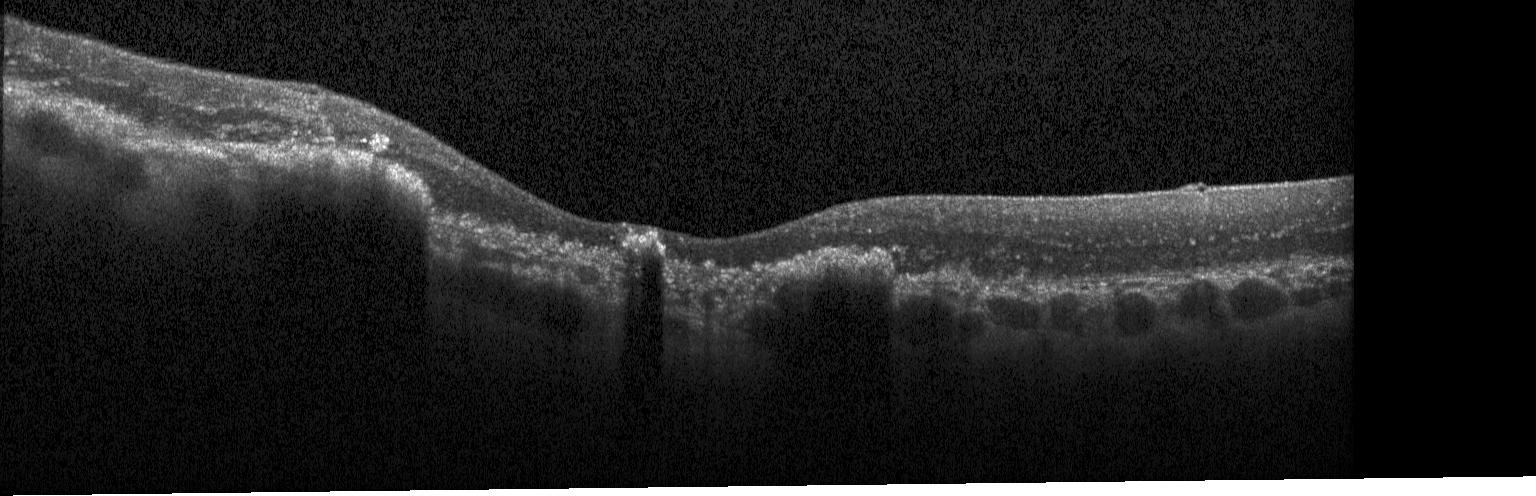
Choroidal neovascularization (CNV).